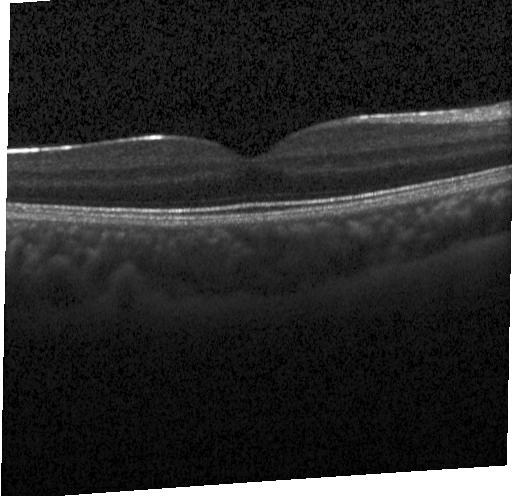

Fovea-centered · Heidelberg Spectralis · retinal OCT B-scan · SD-OCT.
Neither CNV, DME, nor drusen.